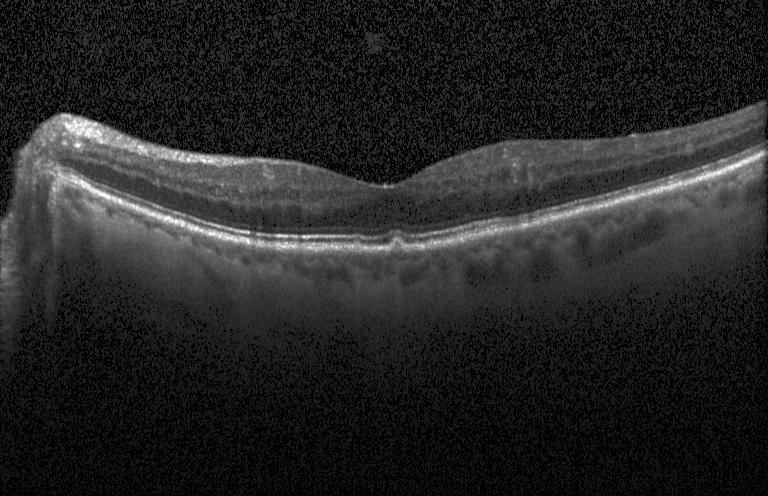 Retinal OCT cross-section showing sub-RPE drusenoid deposits.